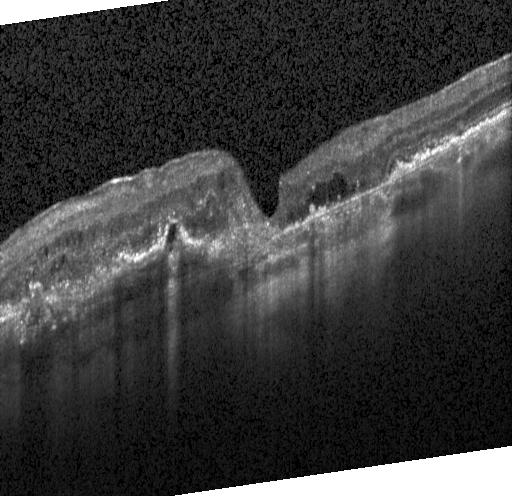

Optical coherence tomography scan. Spectral-domain OCT. Macular scan.
Impression: a choroidal neovascular membrane.